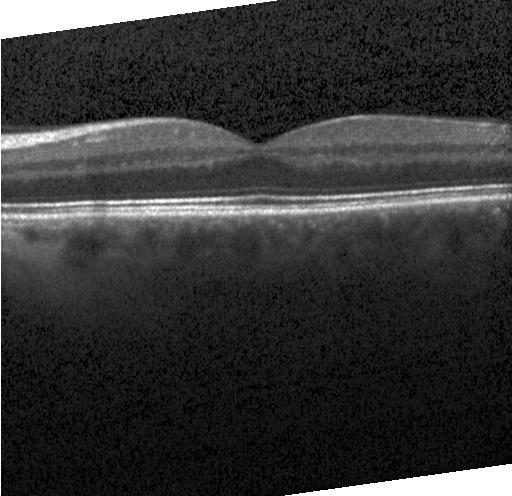

Optical coherence tomography scan. SD-OCT. Instrument: Heidelberg Spectralis. This B-scan demonstrates neither choroidal neovascularization, diabetic macular edema, nor drusen.